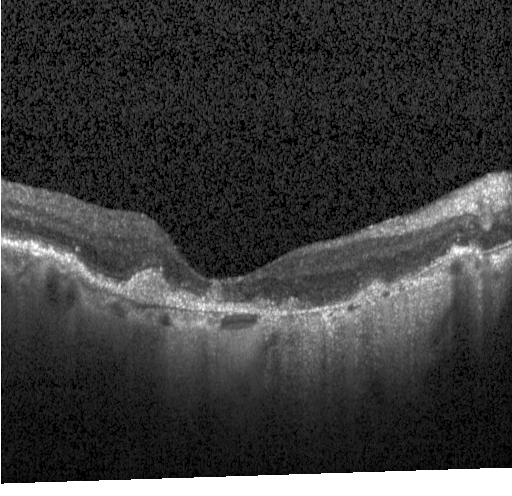
OCT B-scan. Finding: a choroidal neovascular membrane.